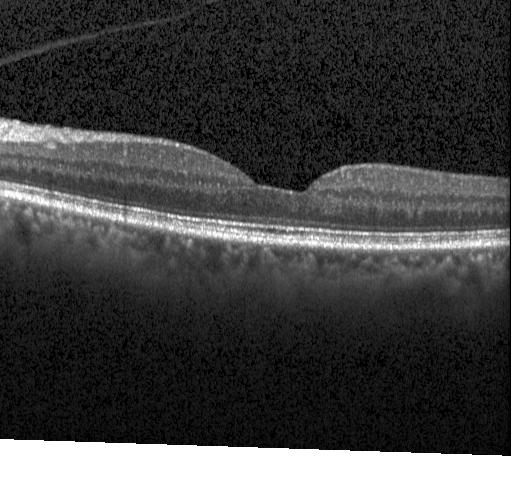

OCT line scan; spectral-domain optical coherence tomography; macular scan; instrument: Heidelberg Spectralis
Assessment: no evidence of CNV, DME, or drusen.